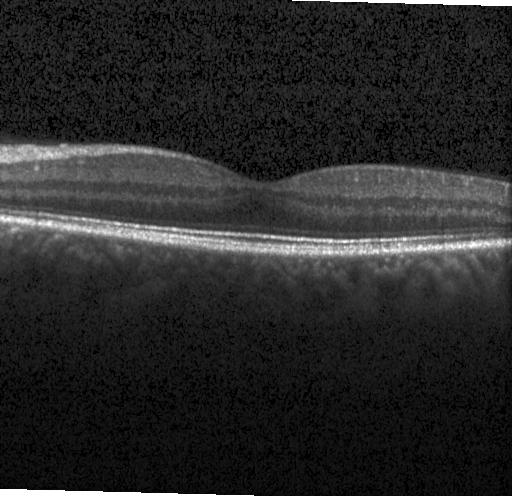
Spectral-domain optical coherence tomography; Heidelberg Spectralis OCT system; optical coherence tomography B-scan. This B-scan demonstrates no evidence of choroidal neovascularization, diabetic macular edema, or drusen.